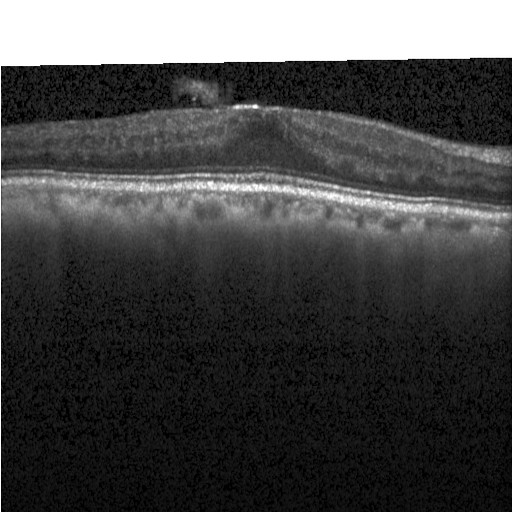
Instrument: Heidelberg Spectralis, OCT B-scan. Finding: diabetic macular edema.